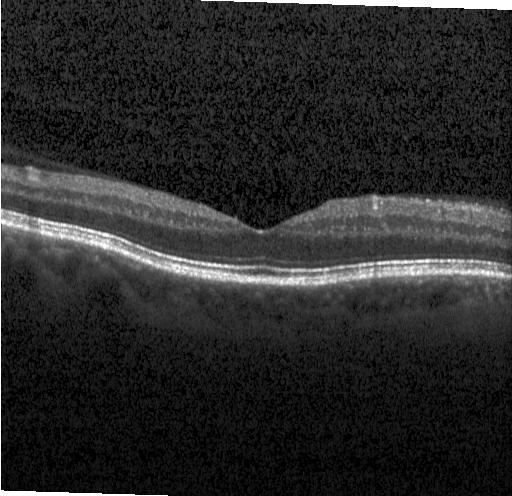

Retinal OCT cross-section; Heidelberg Spectralis OCT system
OCT finding: neither choroidal neovascularization, diabetic macular edema, nor drusen.